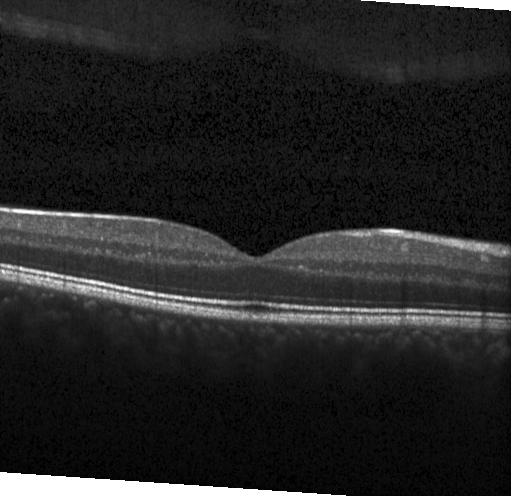

OCT scan showing neither choroidal neovascularization, diabetic macular edema, nor drusen.